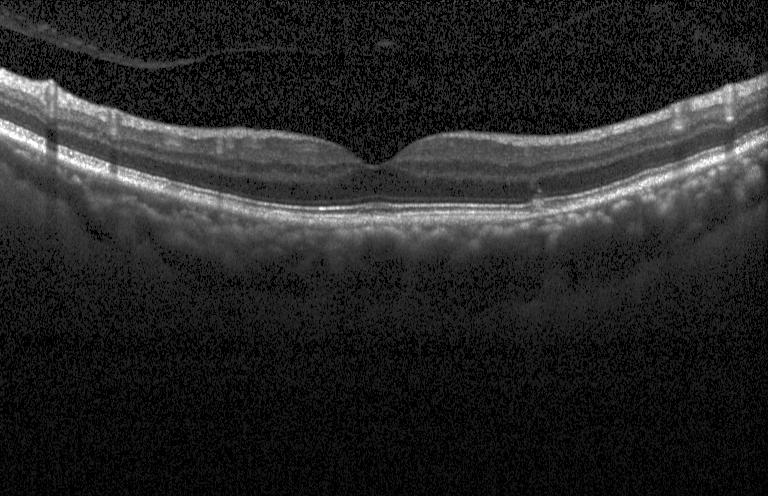 Through the macula · OCT B-scan · Heidelberg Spectralis OCT system — No evidence of choroidal neovascularization, diabetic macular edema, or drusen.